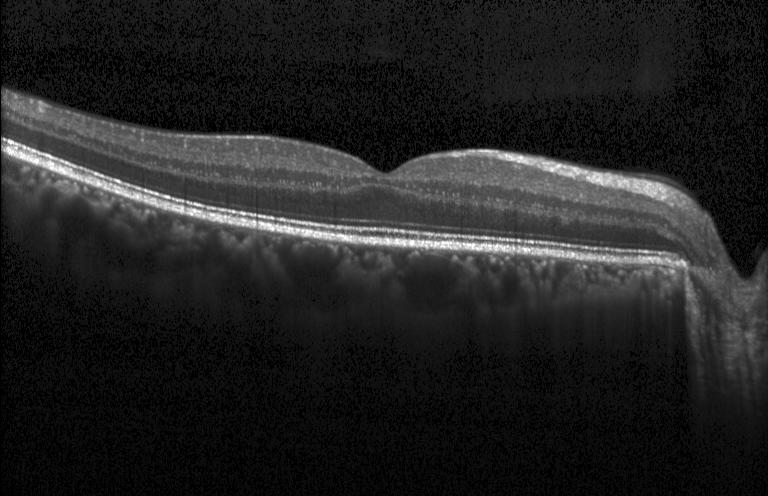
Impression: no choroidal neovascularization, no diabetic macular edema, and no drusen.